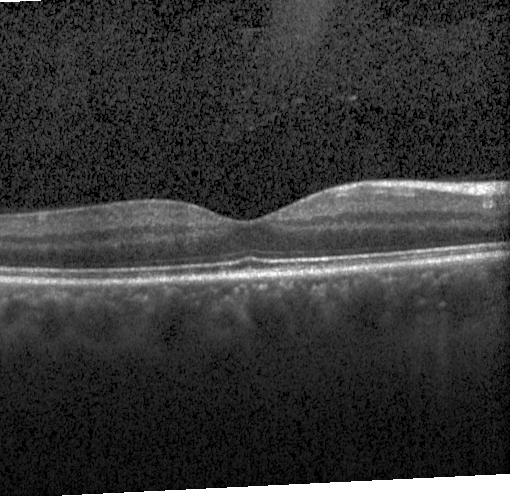
Through the macula · Heidelberg Spectralis OCT system · OCT B-scan.
The scan shows no choroidal neovascularization, diabetic macular edema, or drusen.